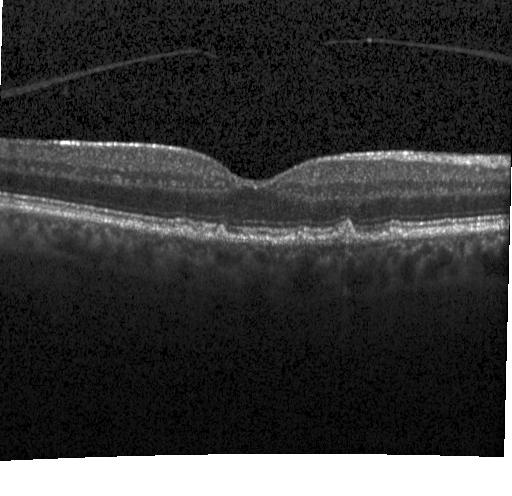
Diagnosis: sub-RPE drusenoid deposits.